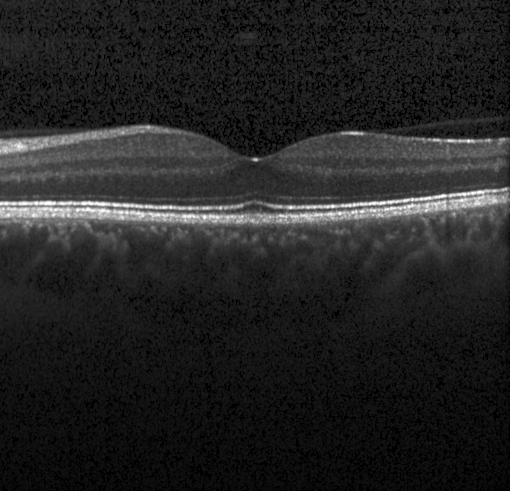

Retinal OCT B-scan — The scan shows no CNV, no DME, and no drusen.